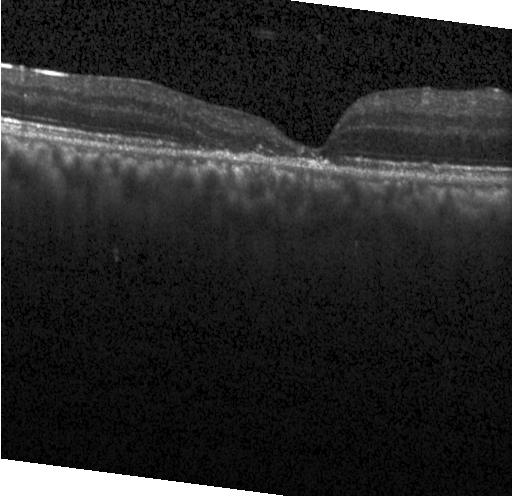
Optical coherence tomography B-scan.
Diagnosis: no evidence of choroidal neovascularization, diabetic macular edema, or drusen.